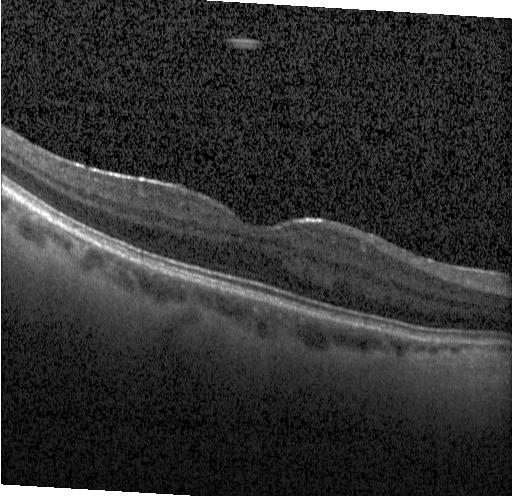

Spectral-domain optical coherence tomography, optical coherence tomography scan, Heidelberg Spectralis OCT system — Neither CNV, DME, nor drusen.